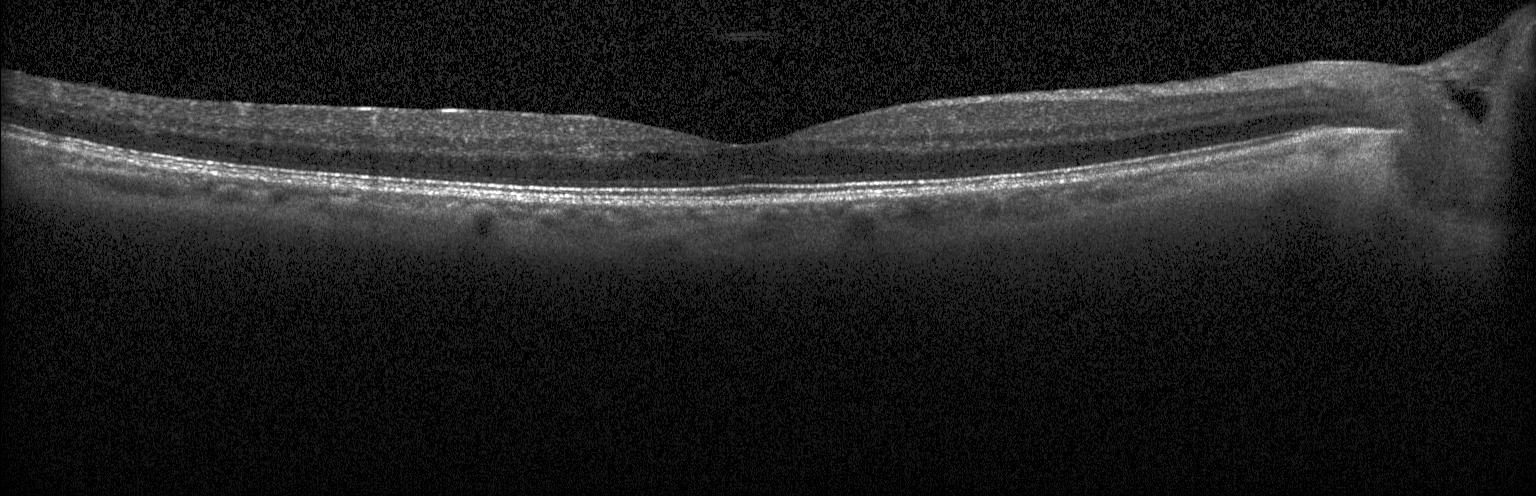 Heidelberg Spectralis OCT system. OCT B-scan. SD-OCT
Diagnosis: no evidence of choroidal neovascularization, diabetic macular edema, or drusen.